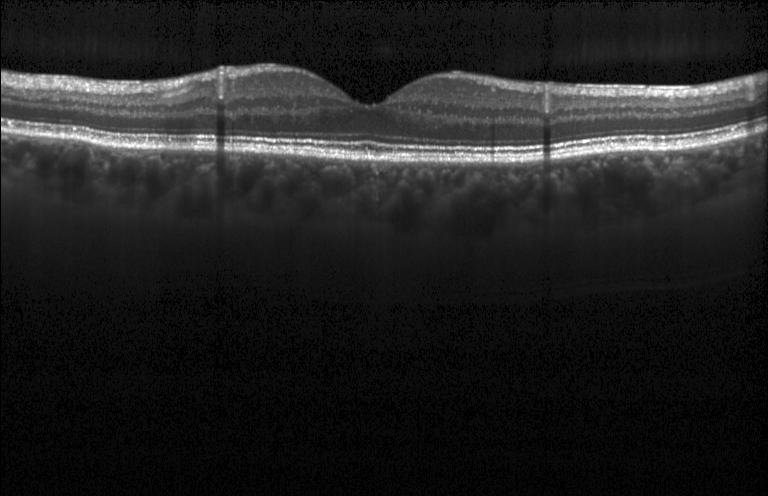
Fovea-centered. Instrument: Heidelberg Spectralis. Spectral-domain optical coherence tomography. Retinal OCT B-scan
OCT finding: no choroidal neovascularization, diabetic macular edema, or drusen.